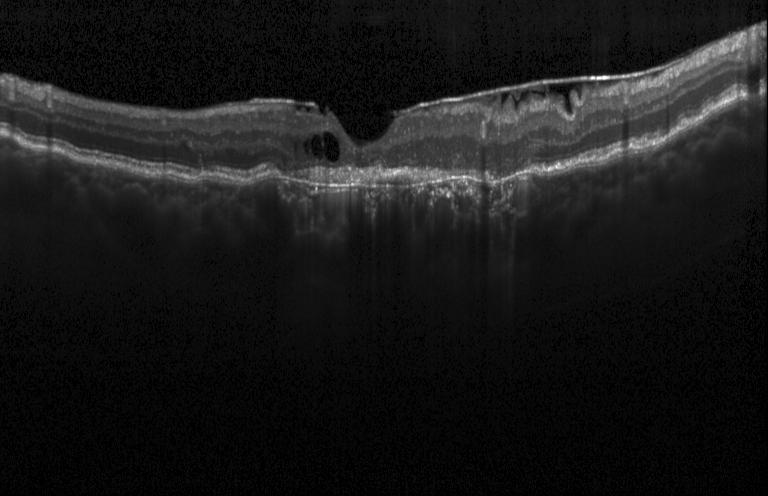 Optical coherence tomography scan; through the macula. The scan shows a choroidal neovascular membrane.